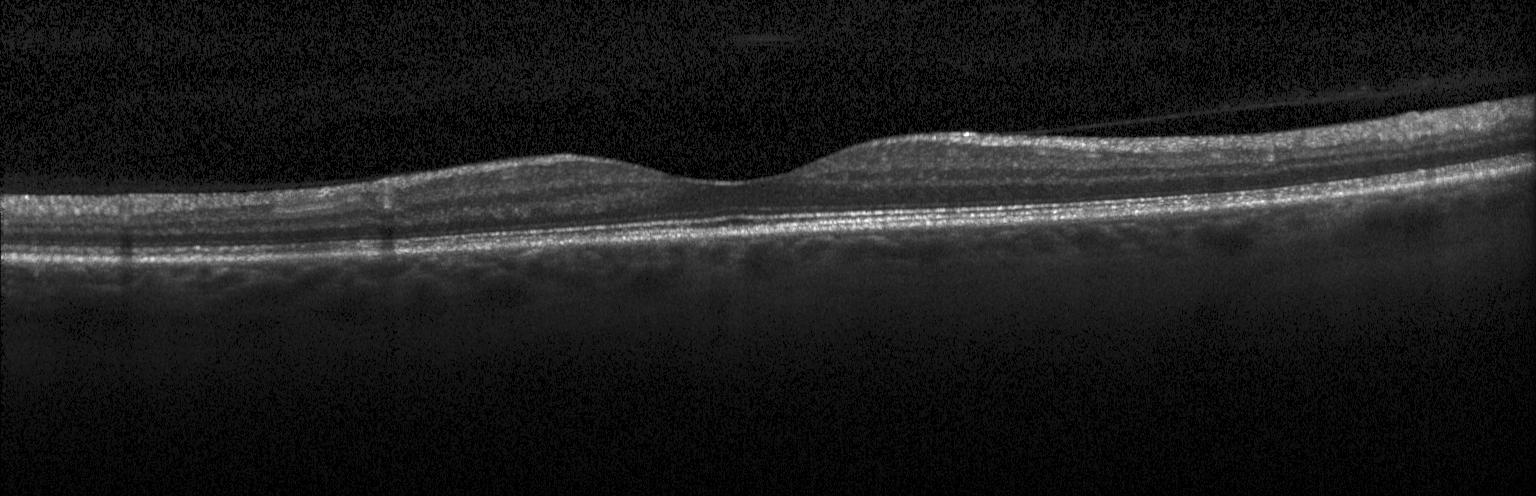
Retinal OCT cross-section
The scan shows no choroidal neovascularization, no diabetic macular edema, and no drusen.